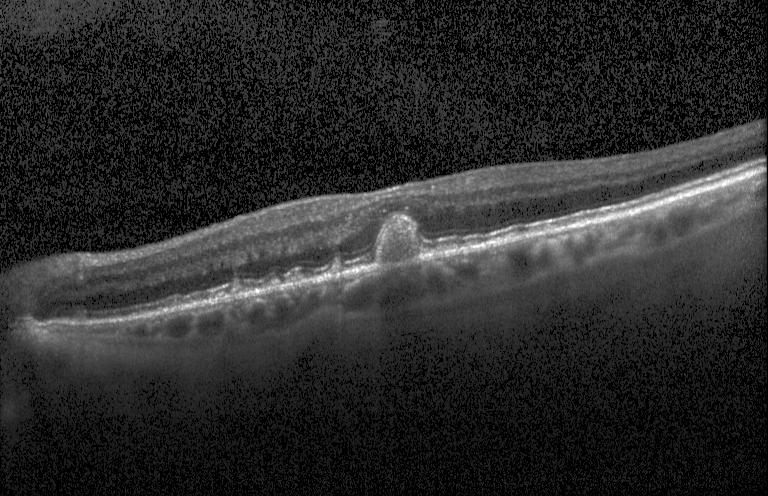

Optical coherence tomography B-scan. Acquired on a Heidelberg Spectralis. Through the macula
Impression: choroidal neovascularization.